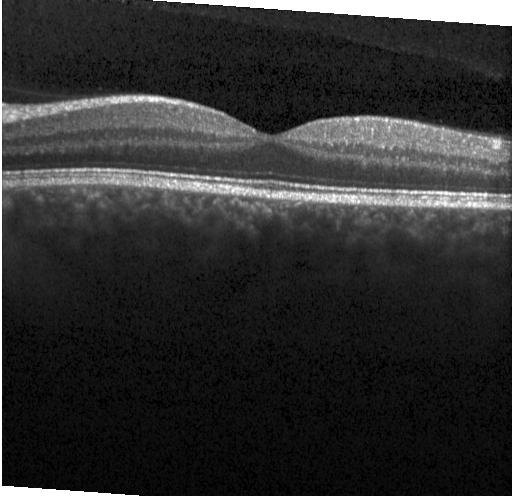
Retinal OCT B-scan · centered on the fovea
The scan shows no CNV, no DME, and no drusen.